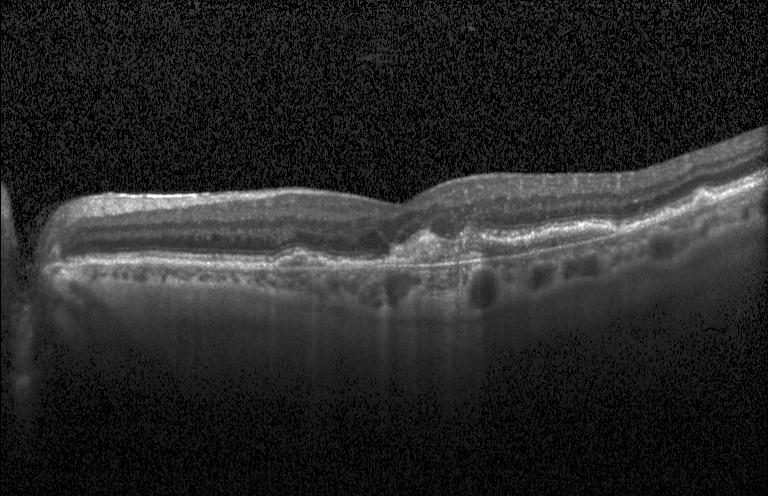

Finding: a choroidal neovascular membrane.